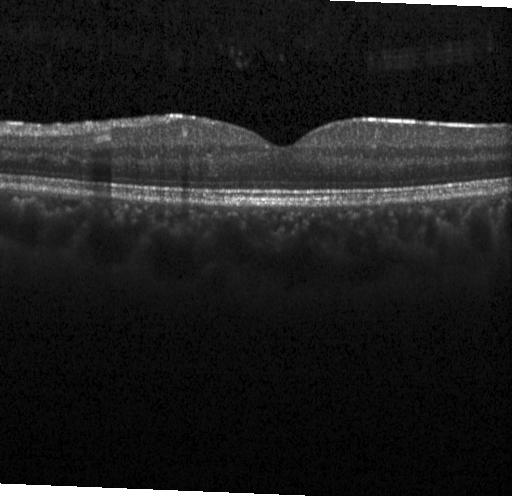 Finding: neither choroidal neovascularization, diabetic macular edema, nor drusen.